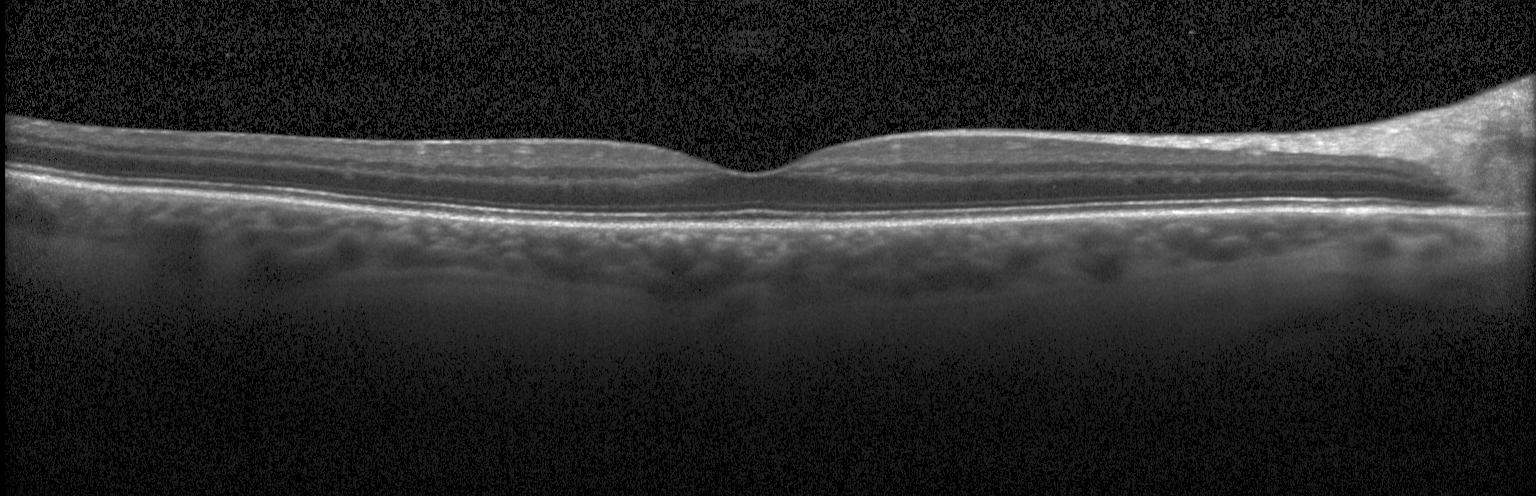 Through the macula. Acquired on a Heidelberg Spectralis. Retinal OCT B-scan. SD-OCT — Assessment: no choroidal neovascularization, no diabetic macular edema, and no drusen.